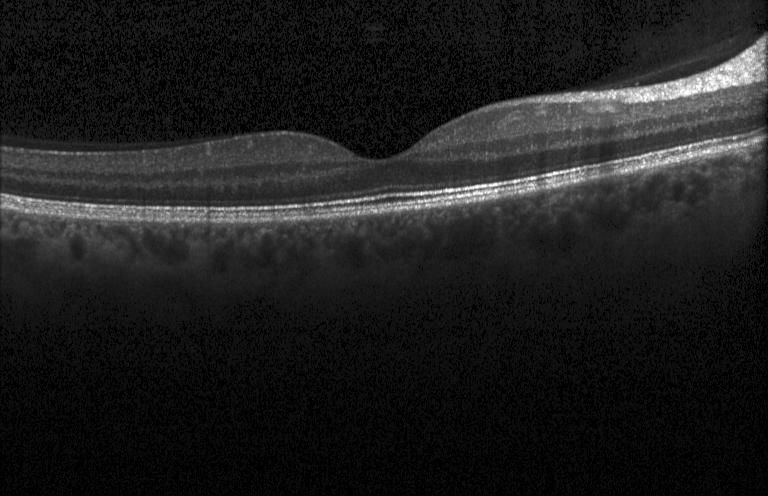

OCT finding: no choroidal neovascularization, no diabetic macular edema, and no drusen.